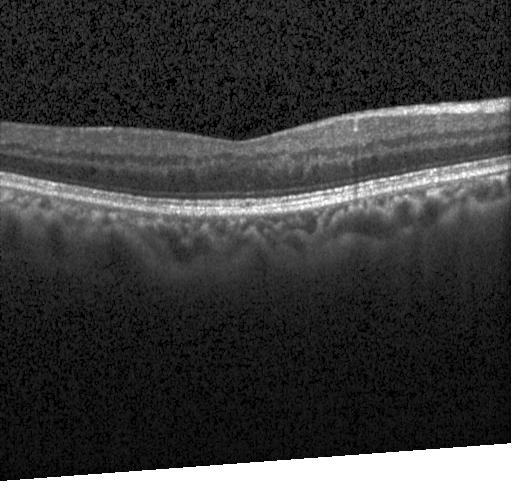
Optical coherence tomography scan — Macular OCT: no choroidal neovascularization, diabetic macular edema, or drusen.